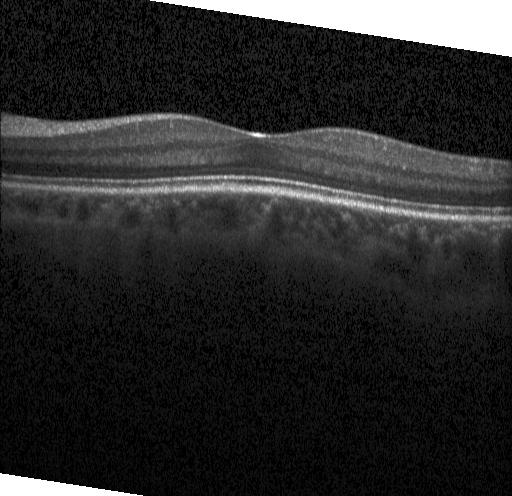
OCT finding: no evidence of choroidal neovascularization, diabetic macular edema, or drusen.